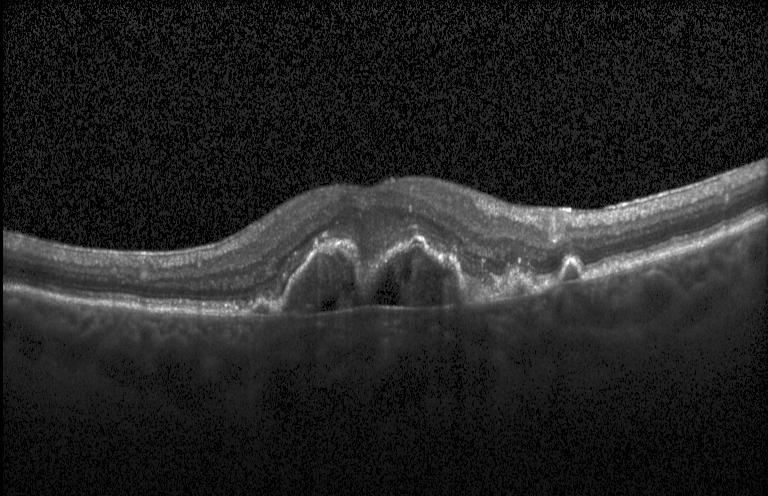
Horizontal scan through the fovea, retinal OCT cross-section
This B-scan demonstrates choroidal neovascularization (CNV).